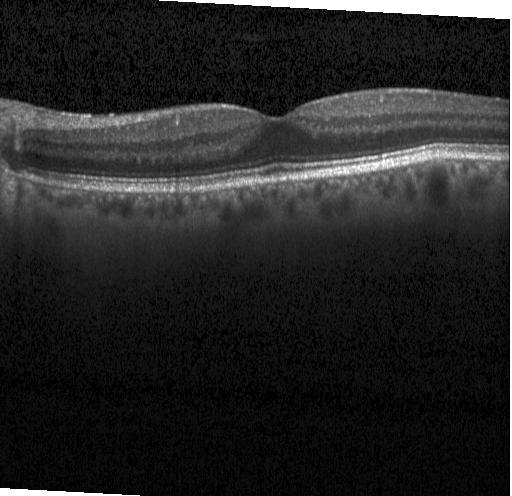 Optical coherence tomography B-scan — Finding: no evidence of choroidal neovascularization, diabetic macular edema, or drusen.